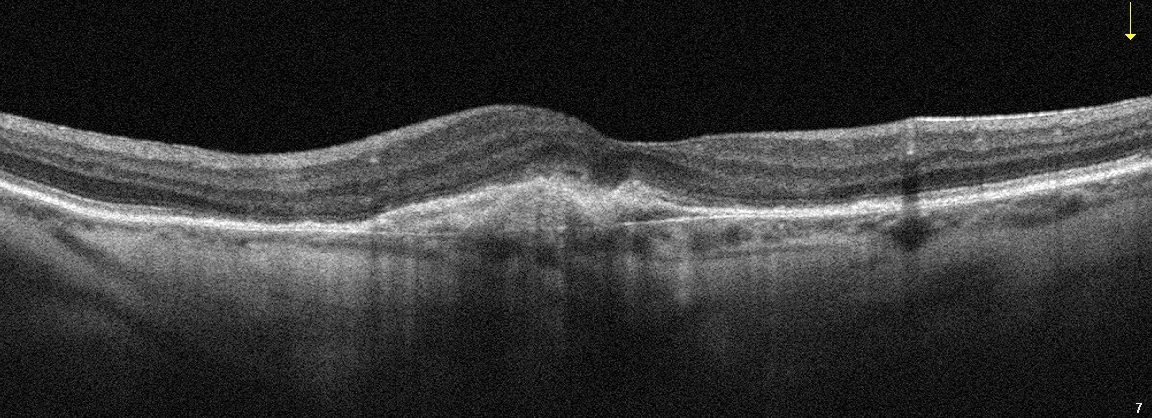 Retinal OCT cross-section. The scan shows age-related macular degeneration.